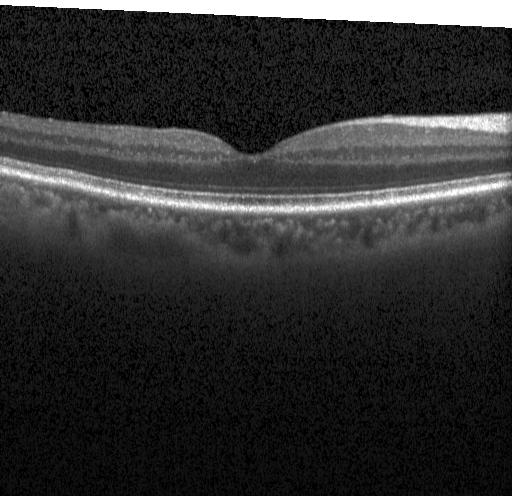 Fovea-centered · OCT line scan · SD-OCT · instrument: Heidelberg Spectralis — Dx: no CNV, DME, or drusen.